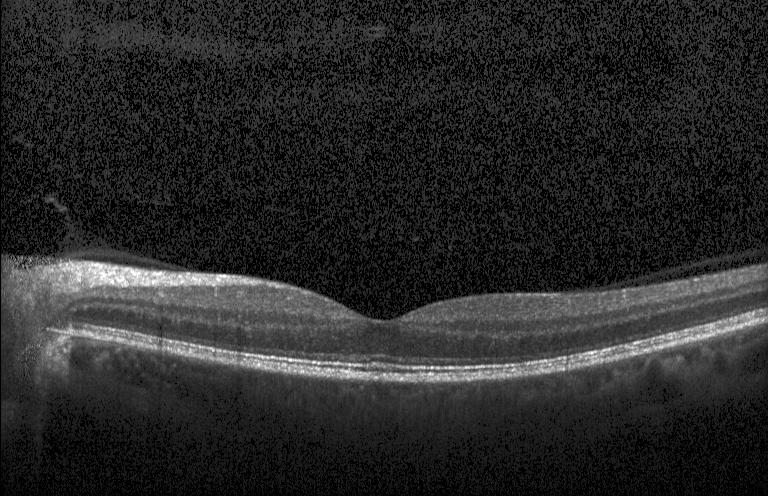
This B-scan demonstrates no CNV, no DME, and no drusen.